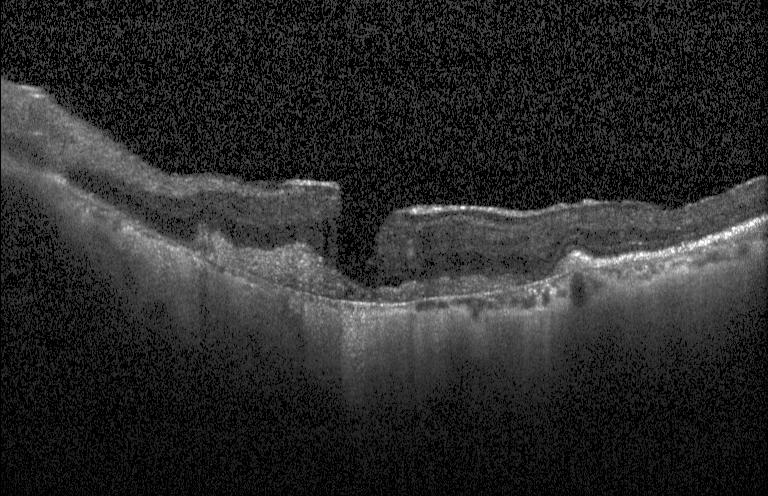
SD-OCT; OCT B-scan; Heidelberg Spectralis
Finding: a choroidal neovascular membrane.